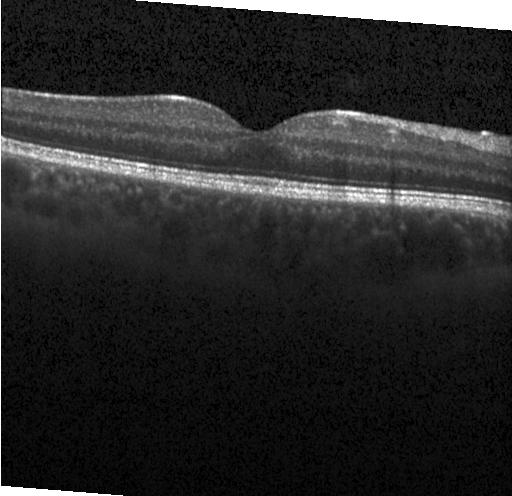 SD-OCT, retinal OCT B-scan, Heidelberg Spectralis OCT system, centered on the fovea — Neither choroidal neovascularization, diabetic macular edema, nor drusen.